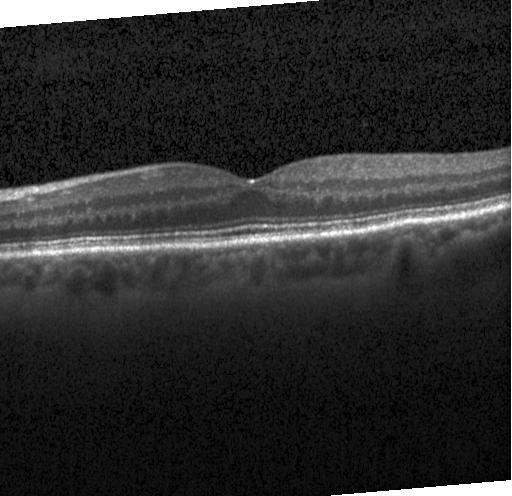
Dx: no evidence of CNV, DME, or drusen.